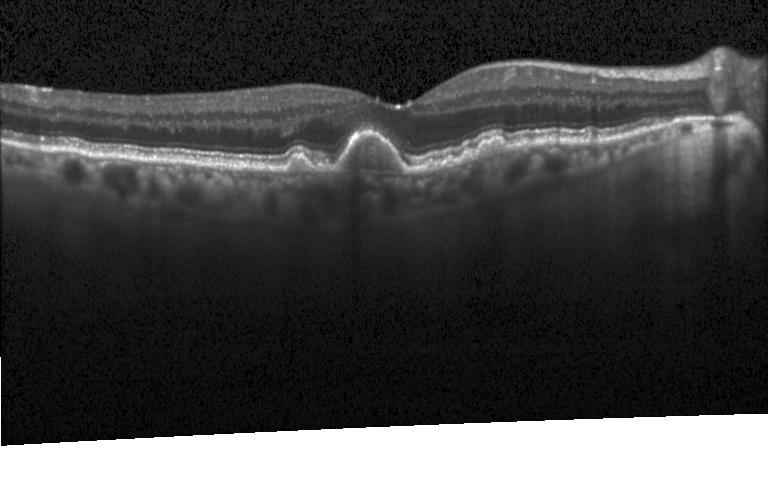

Retinal OCT cross-section.
Finding: sub-RPE drusenoid deposits.